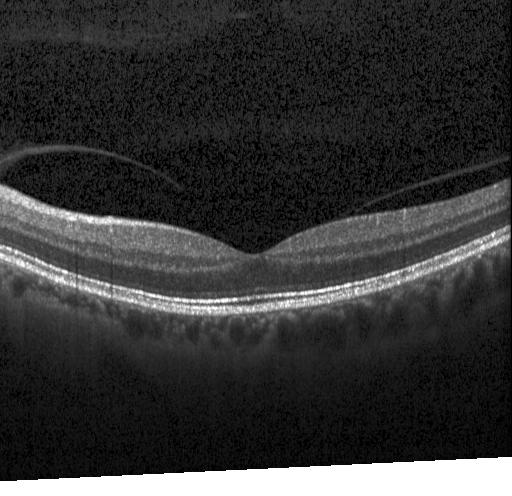
SD-OCT · retinal OCT B-scan · Heidelberg Spectralis OCT system · macular scan — Impression: no choroidal neovascularization, diabetic macular edema, or drusen.